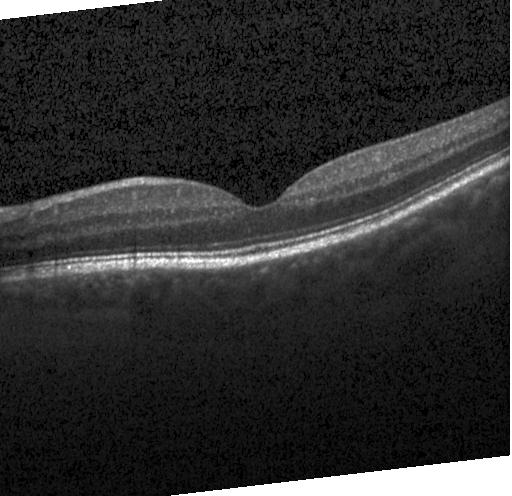
Optical coherence tomography scan — Assessment: no choroidal neovascularization, no diabetic macular edema, and no drusen.